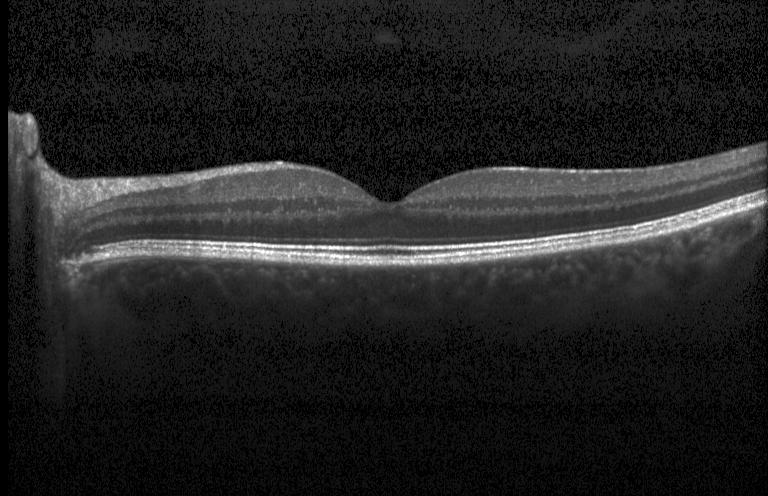

Spectral-domain OCT B-scan: no evidence of CNV, DME, or drusen.